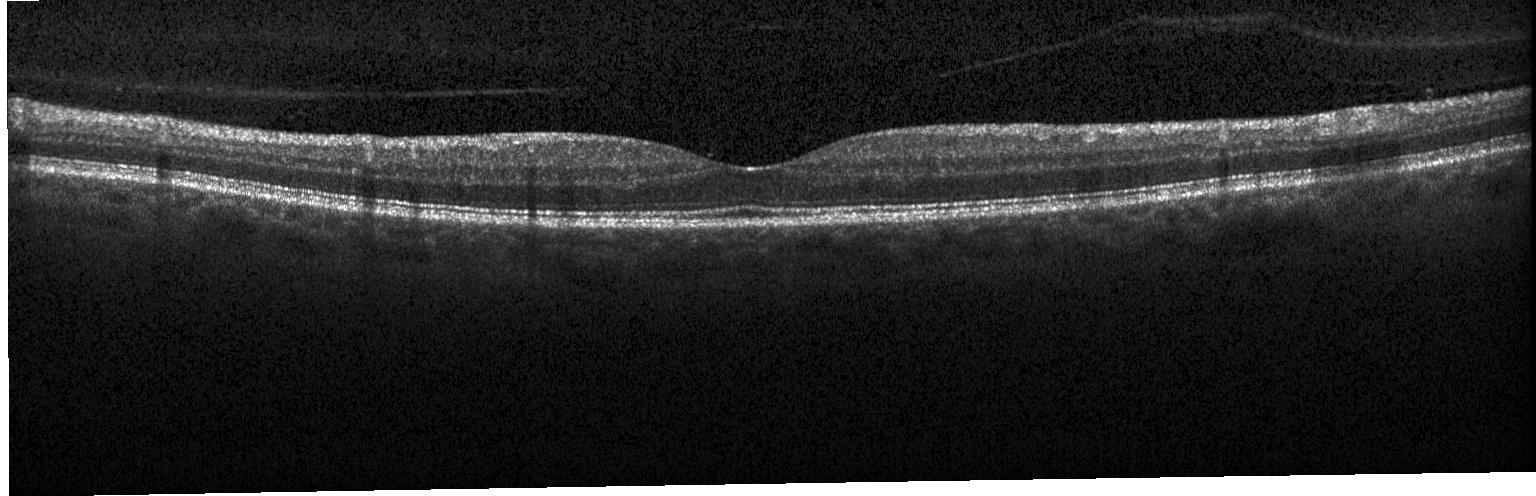 Diagnosis: no evidence of CNV, DME, or drusen.